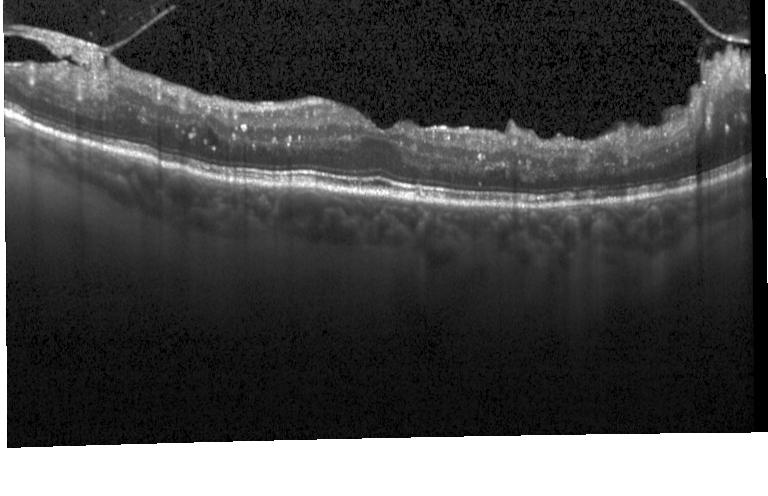 Horizontal scan through the fovea. Heidelberg Spectralis. Optical coherence tomography B-scan. SD-OCT. Impression: DME.